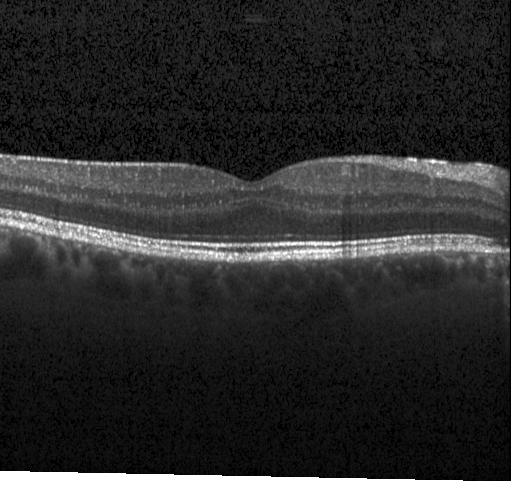

Optical coherence tomography B-scan. Assessment: no choroidal neovascularization, diabetic macular edema, or drusen.